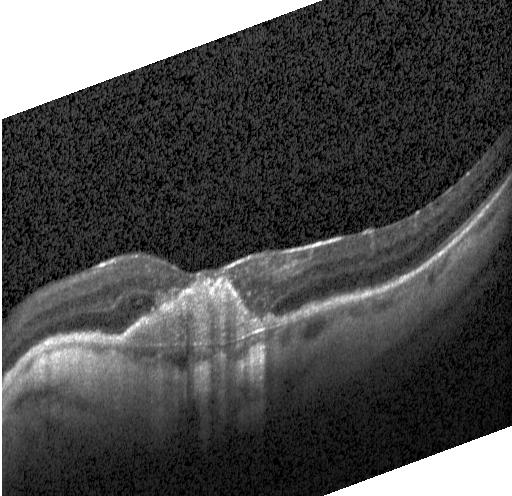

Instrument: Heidelberg Spectralis, retinal OCT B-scan
This B-scan demonstrates a choroidal neovascular membrane.